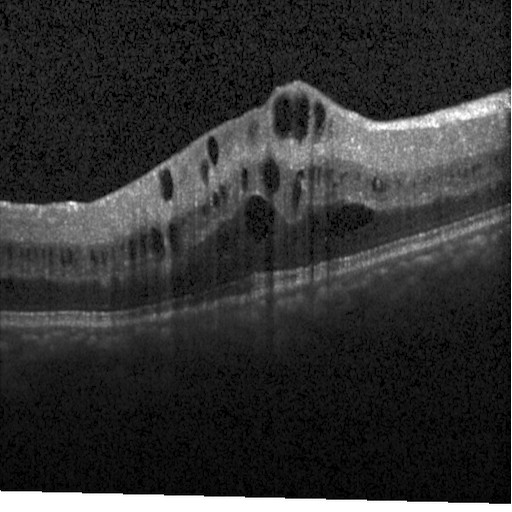
Centered on the fovea; optical coherence tomography B-scan; SD-OCT; Heidelberg Spectralis. Diabetic macular edema.